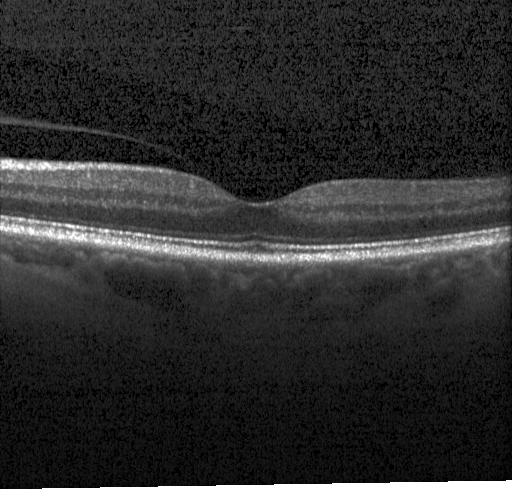 Diagnosis: no evidence of choroidal neovascularization, diabetic macular edema, or drusen.